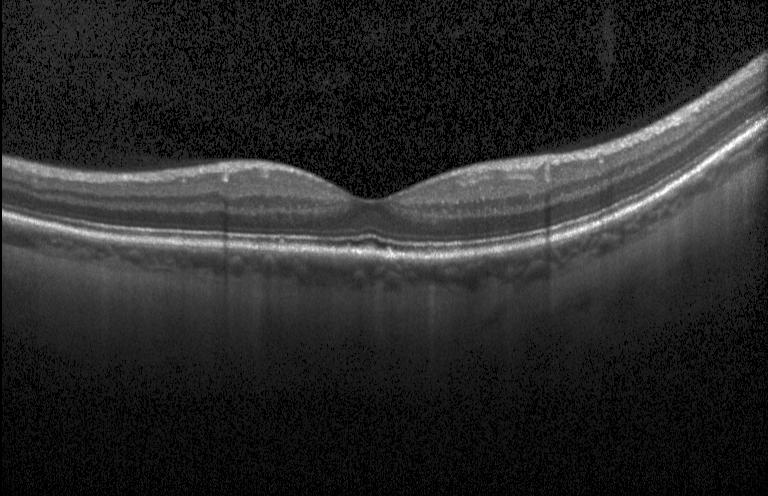
OCT finding: neither choroidal neovascularization, diabetic macular edema, nor drusen.